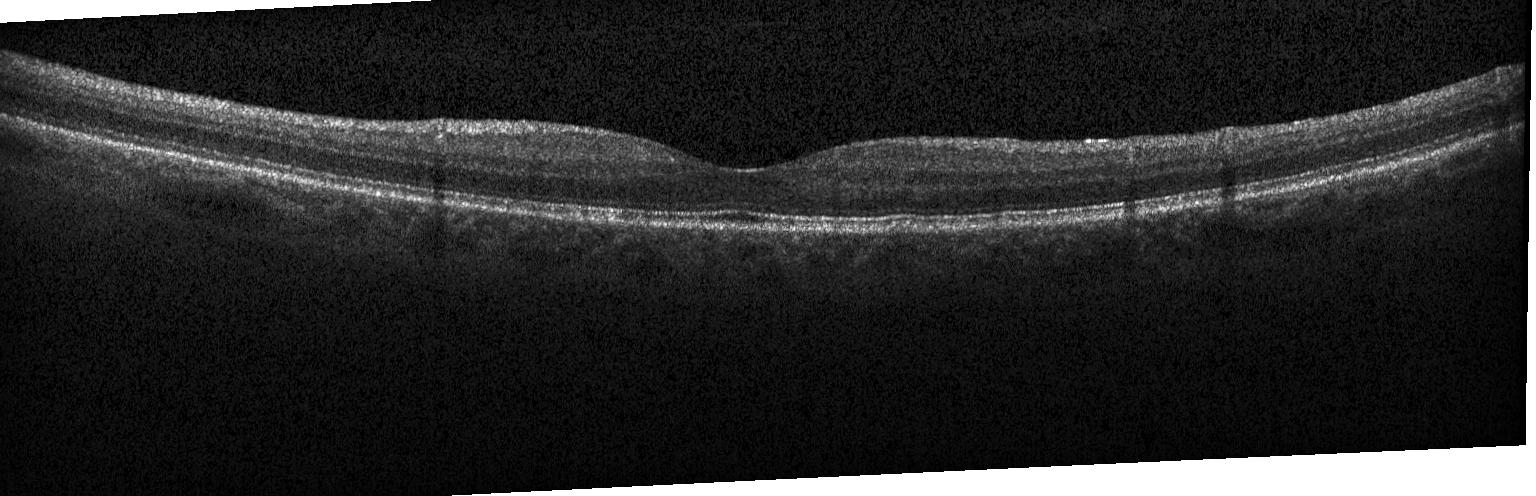

OCT scan showing no choroidal neovascularization, no diabetic macular edema, and no drusen.